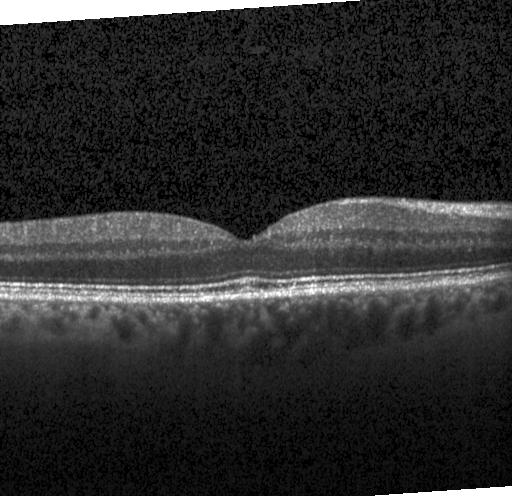 Spectral-domain optical coherence tomography · acquired on a Heidelberg Spectralis · OCT line scan
Macular OCT: no choroidal neovascularization, diabetic macular edema, or drusen.